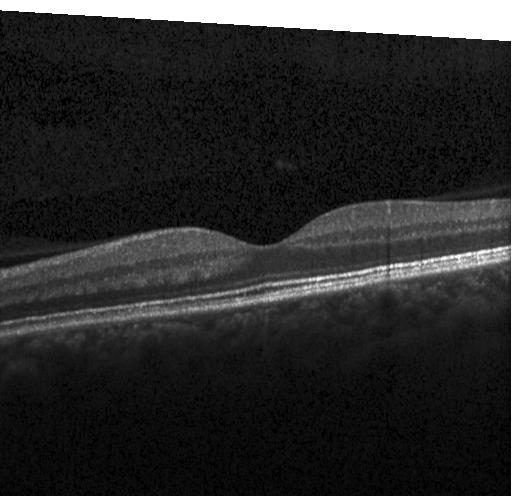
Retinal OCT B-scan, instrument: Heidelberg Spectralis, macular scan, spectral-domain OCT. Diagnosis: no choroidal neovascularization, no diabetic macular edema, and no drusen.